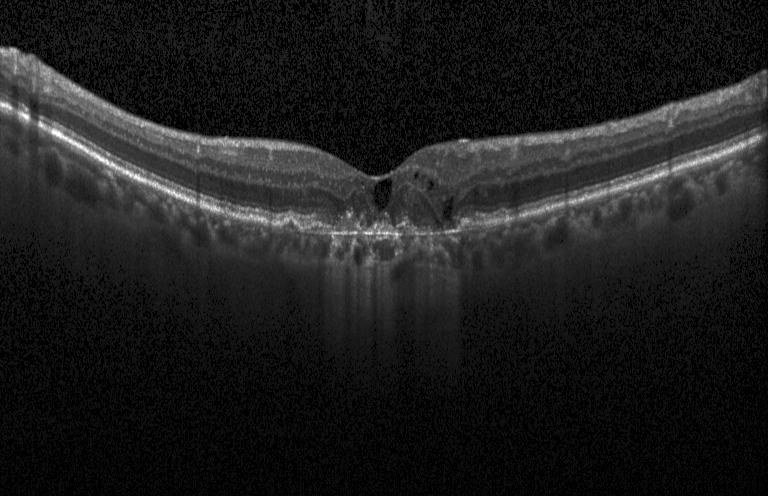

Diagnosis: a choroidal neovascular membrane.